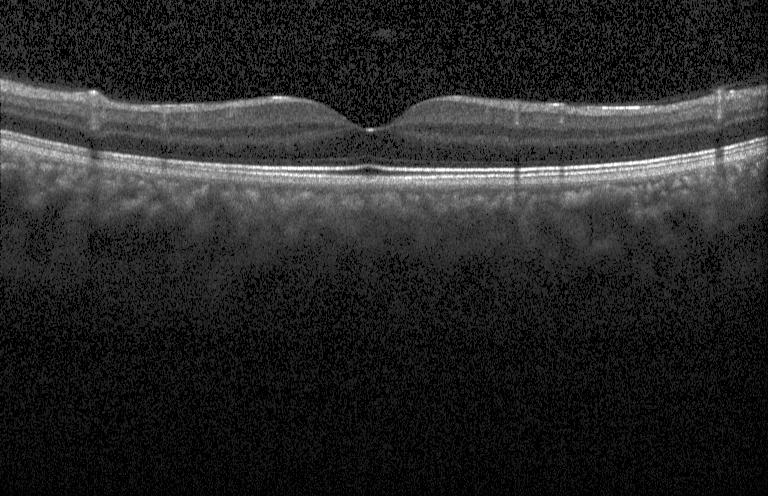

Retinal OCT B-scan. Assessment: no CNV, DME, or drusen.